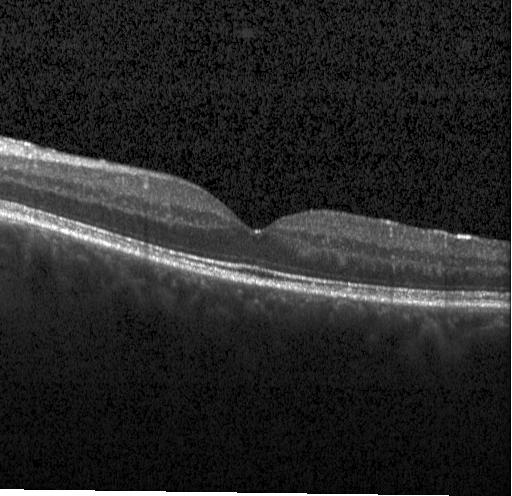

Macular OCT demonstrating no evidence of CNV, DME, or drusen.